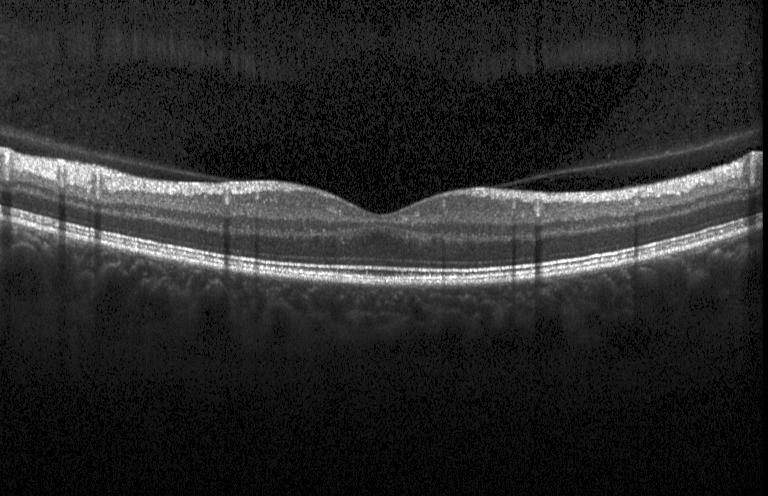

OCT B-scan; horizontal scan through the fovea; spectral-domain optical coherence tomography.
Impression: neither choroidal neovascularization, diabetic macular edema, nor drusen.